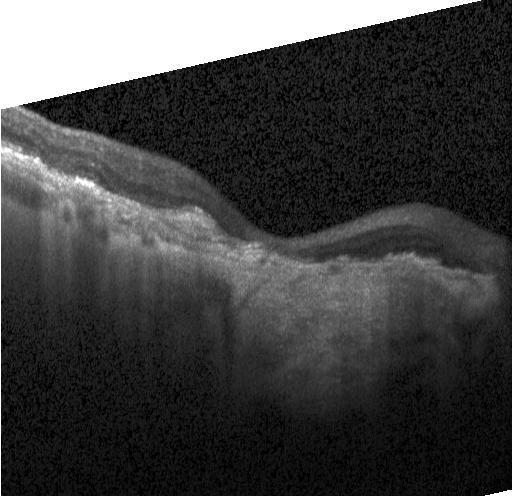
Impression: a choroidal neovascular membrane.